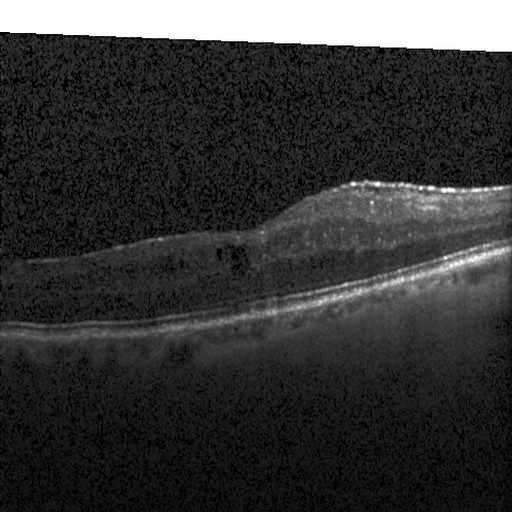
Retinal OCT B-scan. Instrument: Heidelberg Spectralis. Spectral-domain OCT. Centered on the fovea — This B-scan demonstrates DME.